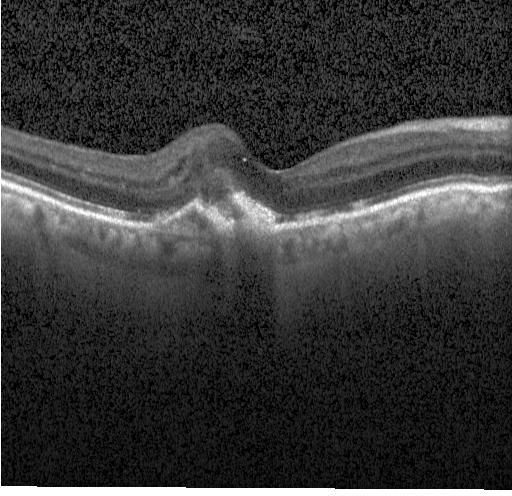
Heidelberg Spectralis. Optical coherence tomography B-scan. Through the macula.
Macular OCT: CNV.